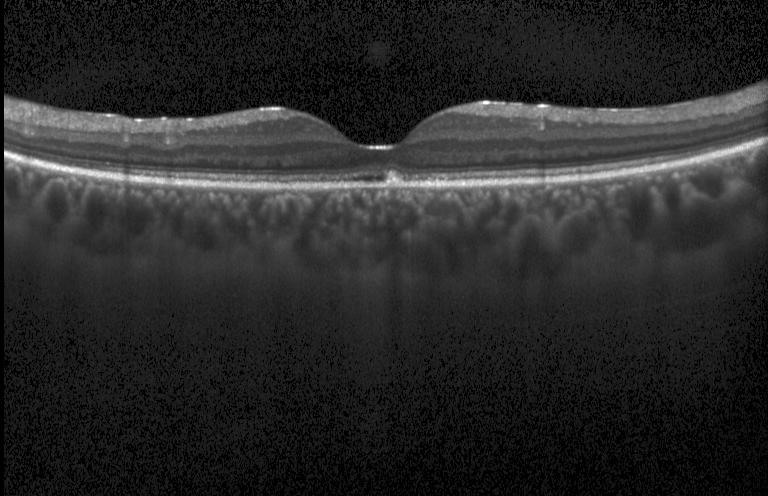
Retinal OCT cross-section.
The scan shows no choroidal neovascularization, diabetic macular edema, or drusen.